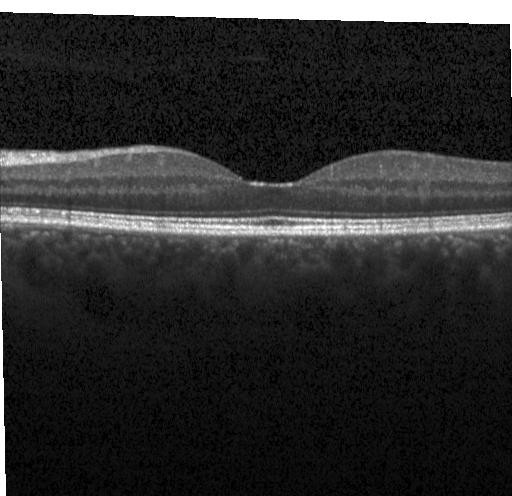
Optical coherence tomography scan; SD-OCT; fovea-centered.
OCT finding: no choroidal neovascularization, diabetic macular edema, or drusen.